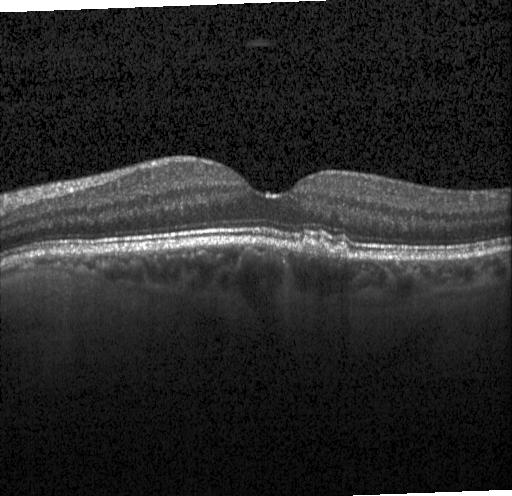
Drusen.